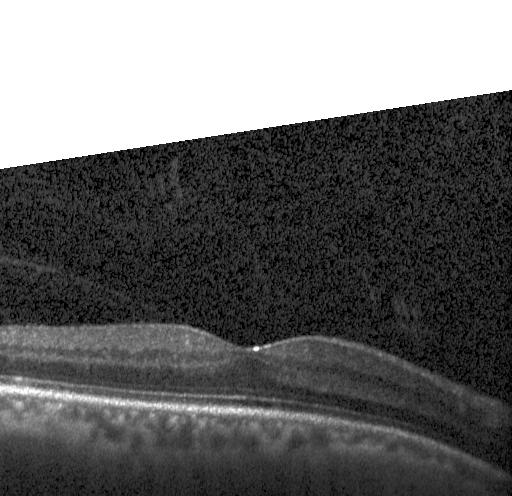 Optical coherence tomography scan. SD-OCT. Heidelberg Spectralis OCT system
Assessment: neither choroidal neovascularization, diabetic macular edema, nor drusen.